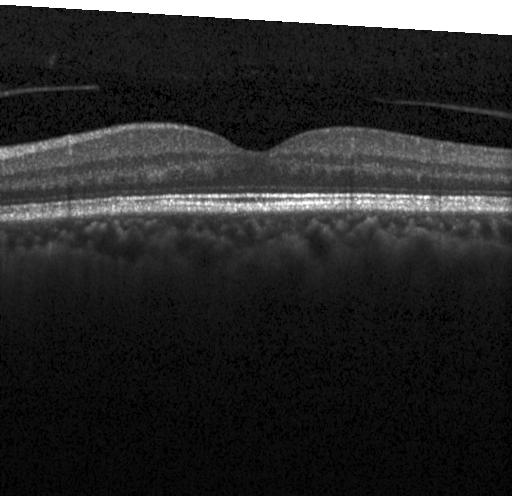

OCT B-scan — OCT finding: neither choroidal neovascularization, diabetic macular edema, nor drusen.